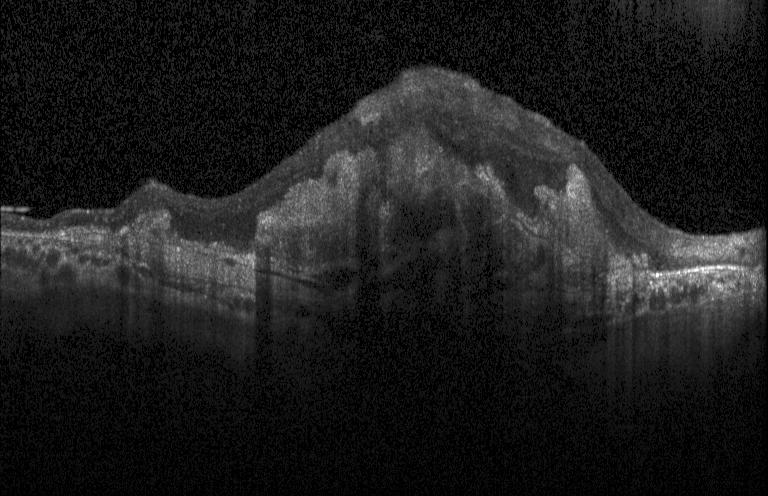
Optical coherence tomography B-scan
Diagnosis: choroidal neovascularization (CNV).